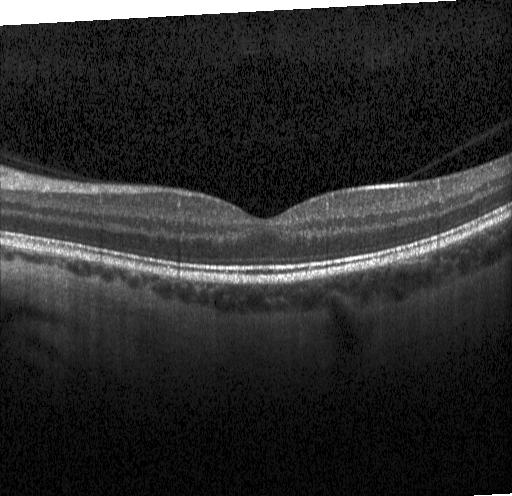 Spectral-domain OCT B-scan: neither choroidal neovascularization, diabetic macular edema, nor drusen.